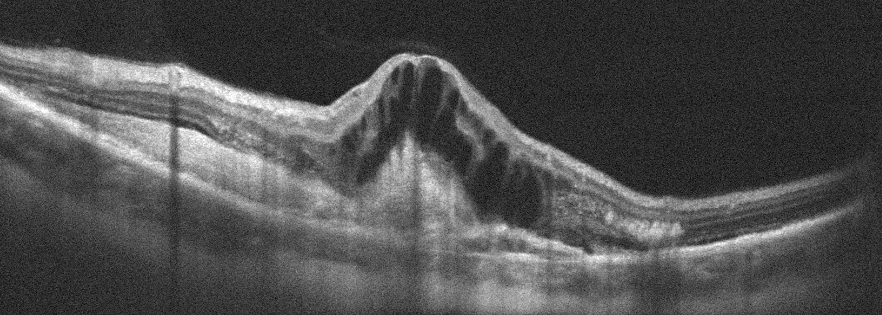
OCT B-scan. Instrument: Optovue Avanti RTVue XR — Finding: AMD.